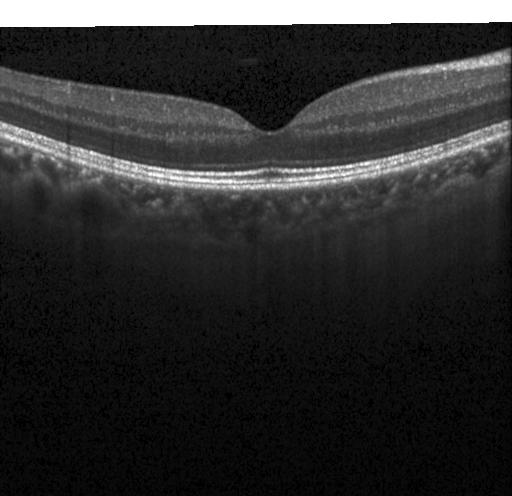 Spectral-domain OCT, optical coherence tomography scan, acquired on a Heidelberg Spectralis — Dx: no choroidal neovascularization, diabetic macular edema, or drusen.